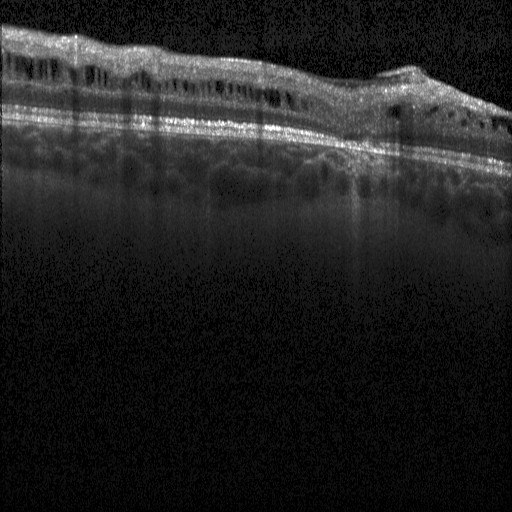

Spectral-domain optical coherence tomography; centered on the fovea; Heidelberg Spectralis; optical coherence tomography B-scan.
The scan shows diabetic macular edema (DME).